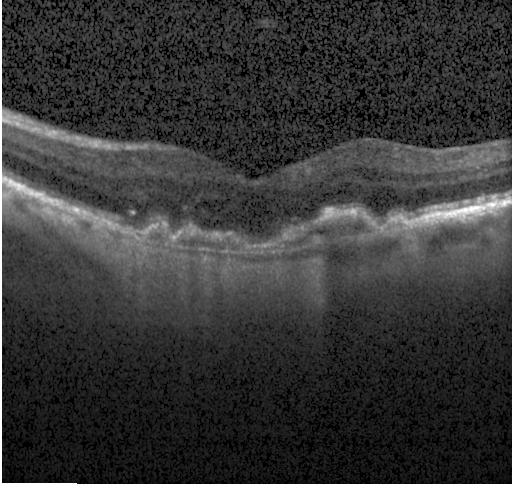
OCT B-scan, instrument: Heidelberg Spectralis
Diagnosis: a choroidal neovascular membrane.